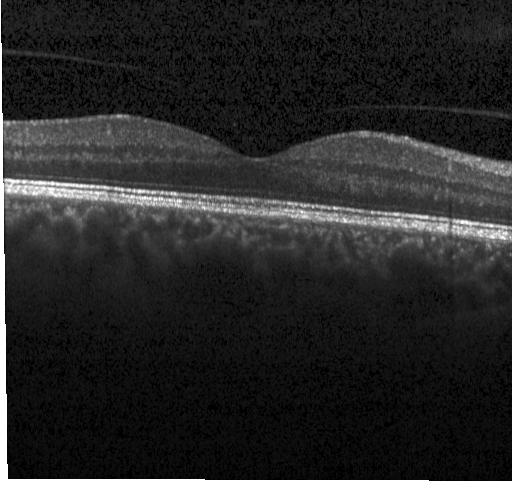
OCT scan showing no CNV, no DME, and no drusen.